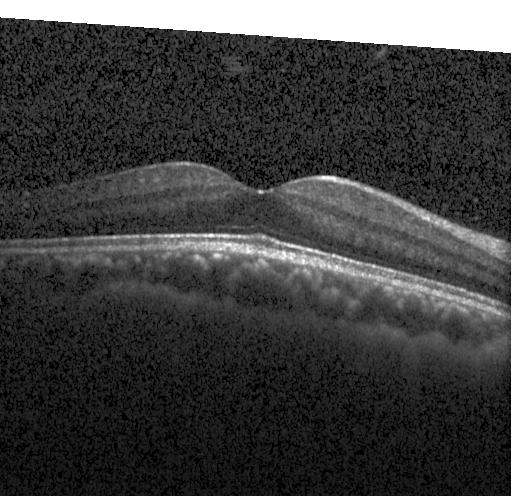
Impression: no CNV, no DME, and no drusen.